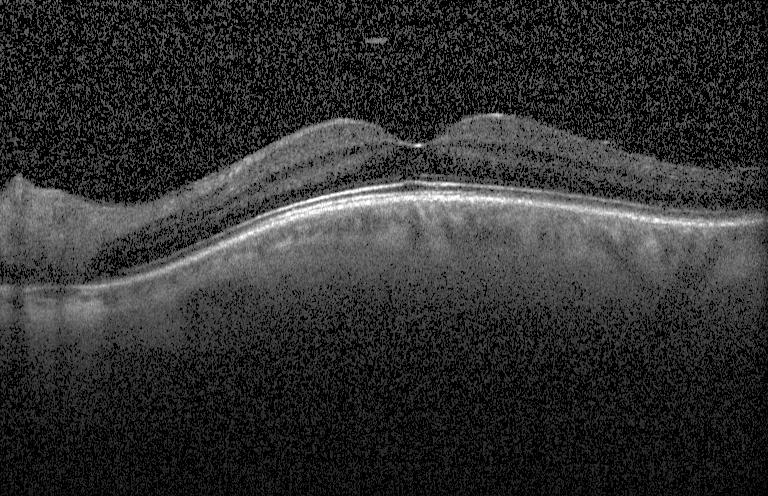

Heidelberg Spectralis; optical coherence tomography scan
Macular OCT: neither CNV, DME, nor drusen.